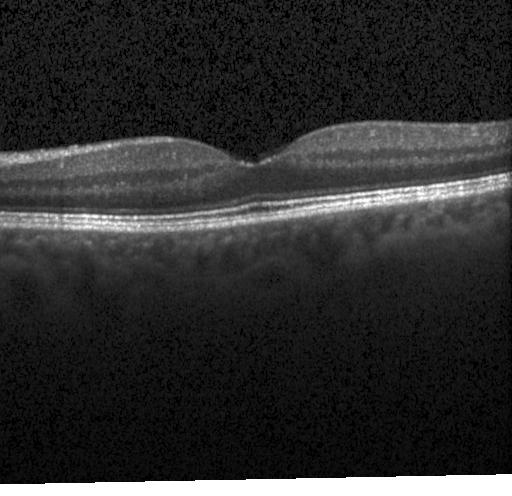
Optical coherence tomography scan; spectral-domain OCT; horizontal scan through the fovea; instrument: Heidelberg Spectralis
Assessment: neither choroidal neovascularization, diabetic macular edema, nor drusen.